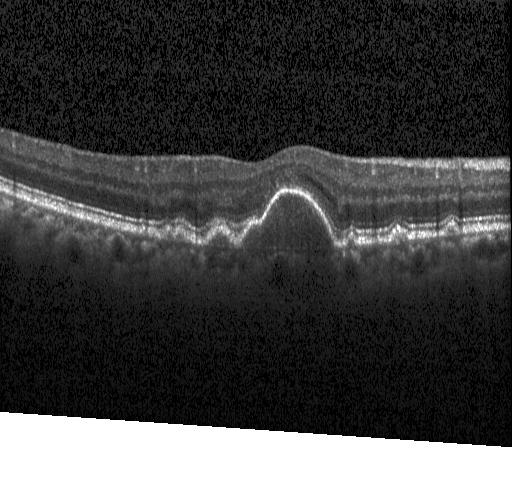
OCT line scan — Finding: multiple drusen.